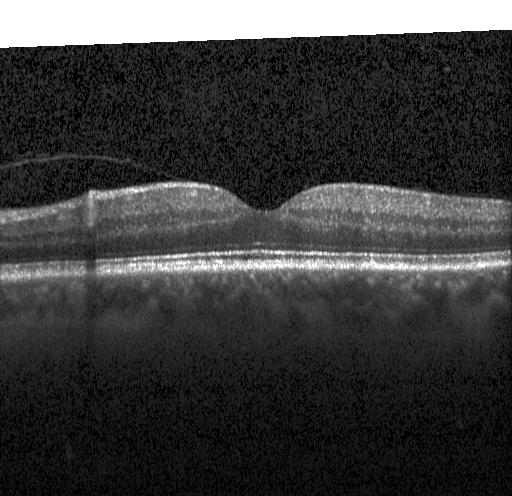

Retinal OCT B-scan. This B-scan demonstrates no choroidal neovascularization, no diabetic macular edema, and no drusen.